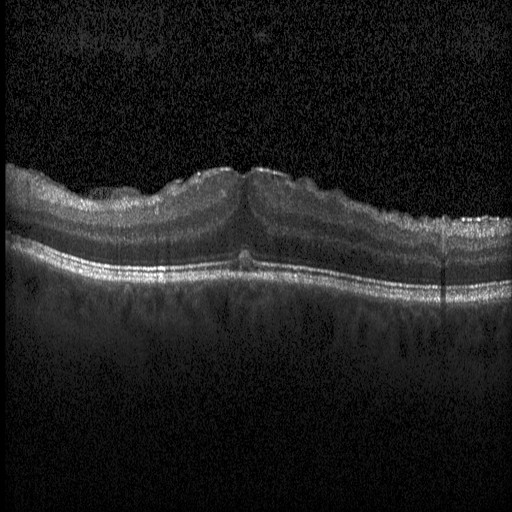 Spectral-domain OCT · optical coherence tomography B-scan — DME.